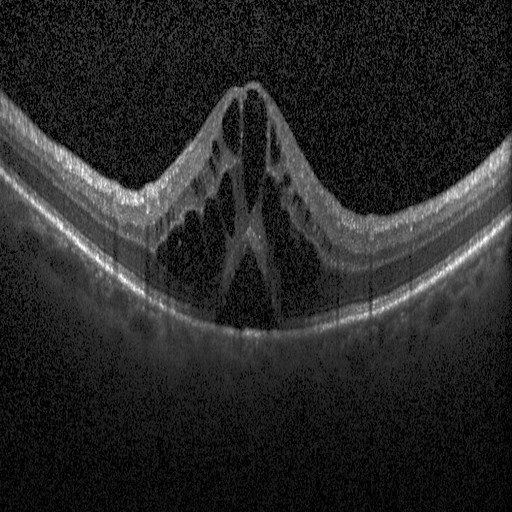

Optical coherence tomography B-scan. Finding: diabetic macular edema.